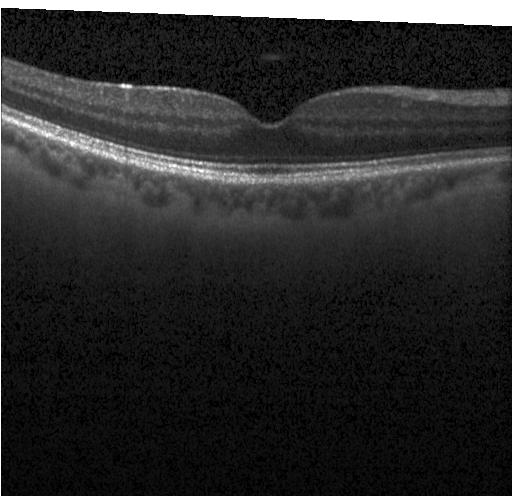

Fovea-centered, retinal OCT B-scan, acquired on a Heidelberg Spectralis, spectral-domain OCT. Impression: no evidence of choroidal neovascularization, diabetic macular edema, or drusen.